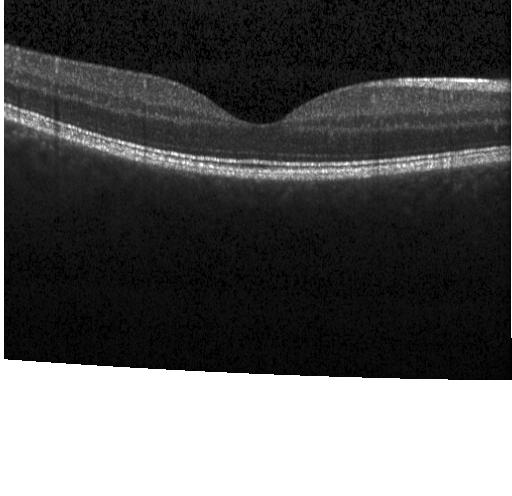 Dx: no evidence of choroidal neovascularization, diabetic macular edema, or drusen.